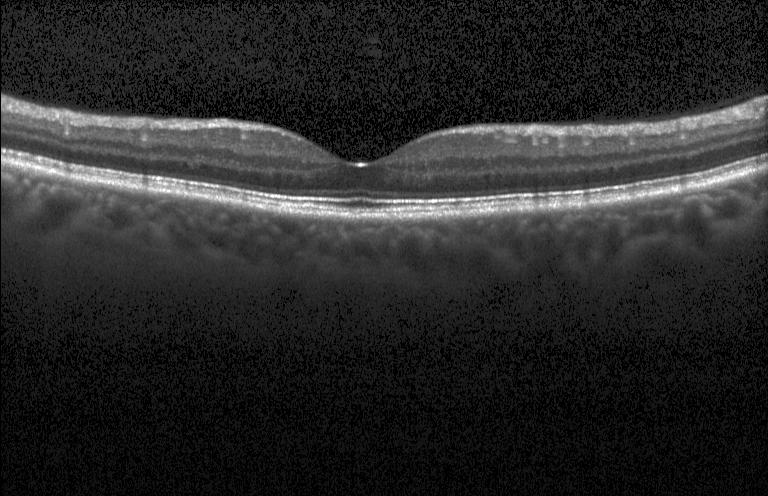 Optical coherence tomography B-scan — Diagnosis: neither CNV, DME, nor drusen.